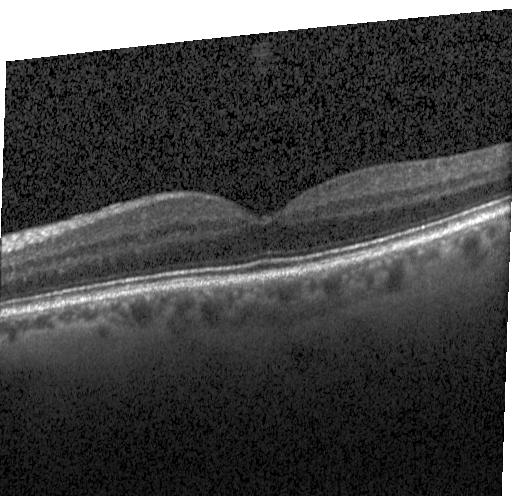 Optical coherence tomography B-scan.
The scan shows no choroidal neovascularization, no diabetic macular edema, and no drusen.